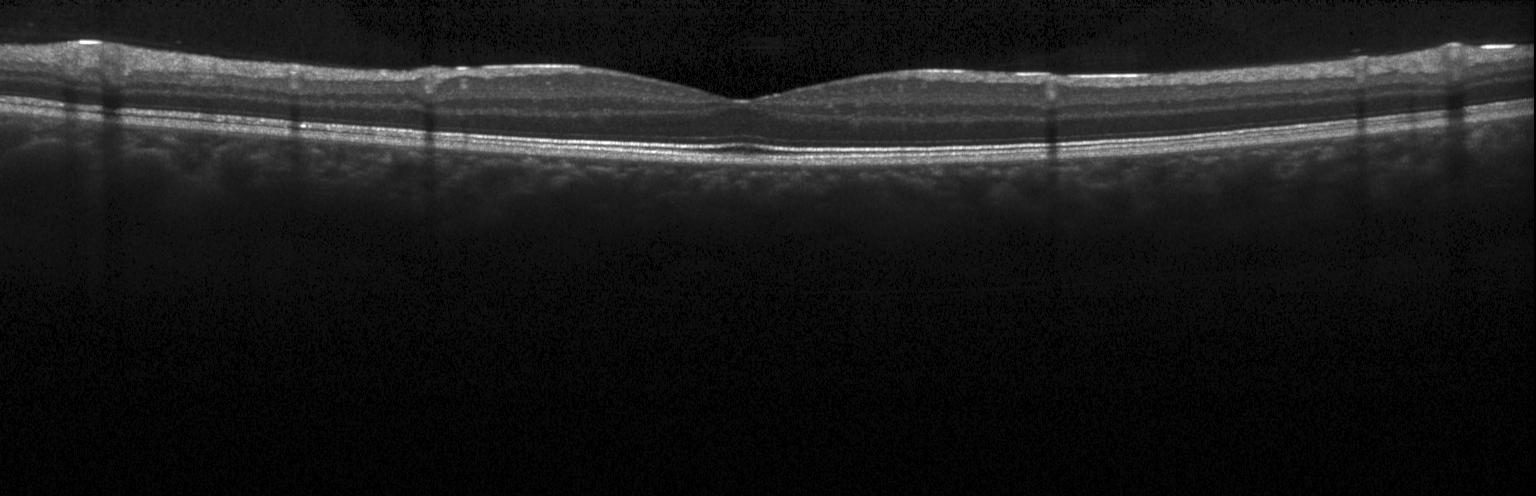

Finding: no choroidal neovascularization, diabetic macular edema, or drusen.